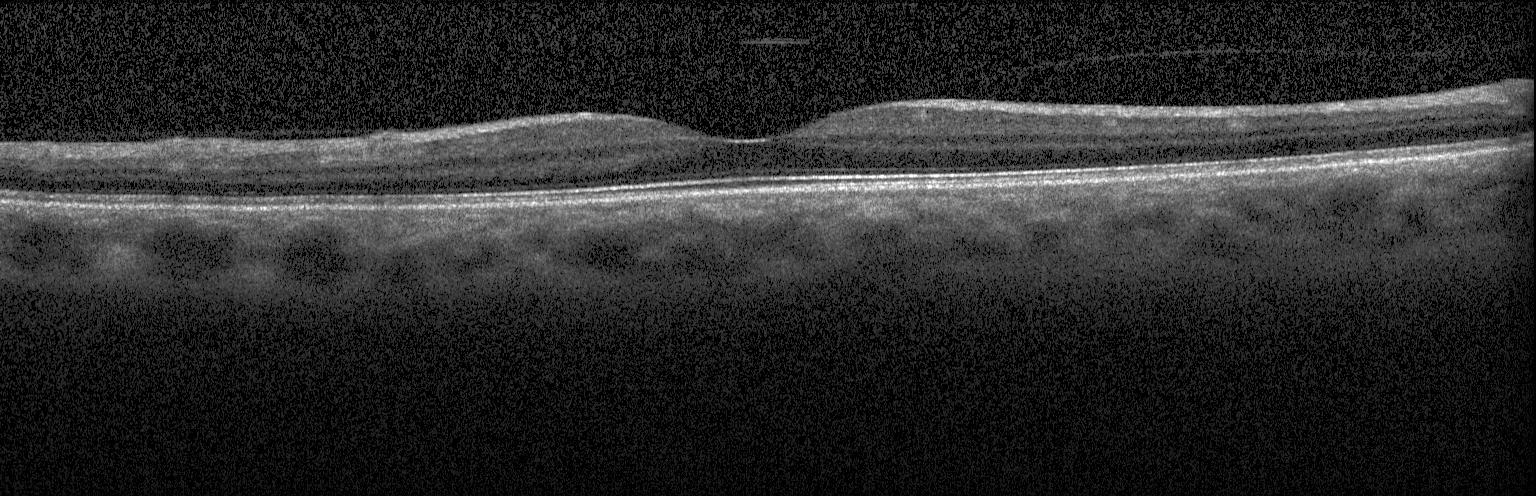

Assessment: neither CNV, DME, nor drusen.